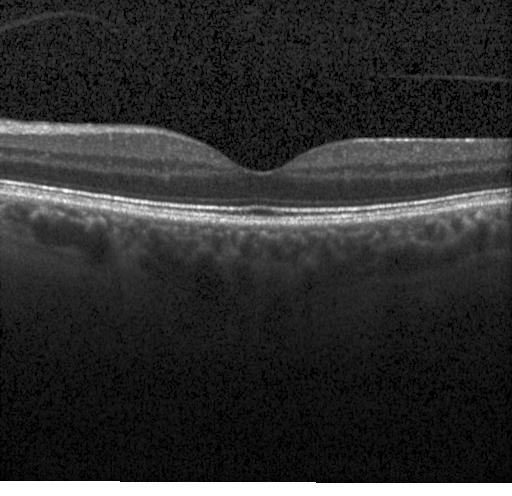 Instrument: Heidelberg Spectralis. Centered on the fovea. Optical coherence tomography B-scan — Dx: neither choroidal neovascularization, diabetic macular edema, nor drusen.